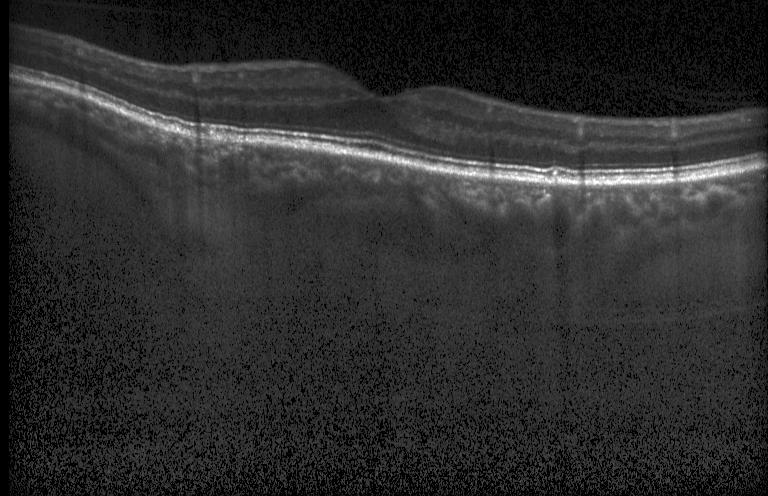 Neither choroidal neovascularization, diabetic macular edema, nor drusen.